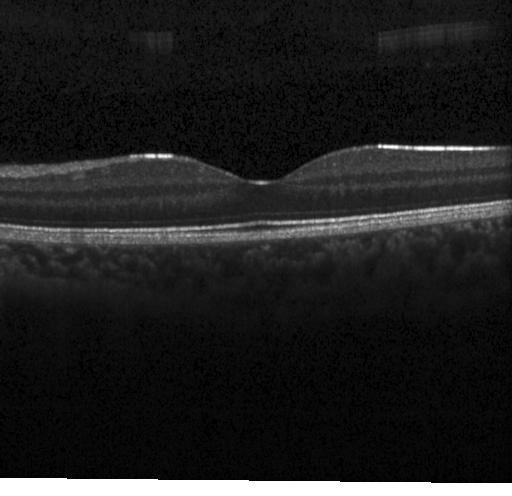 Retinal OCT B-scan
Impression: no choroidal neovascularization, no diabetic macular edema, and no drusen.